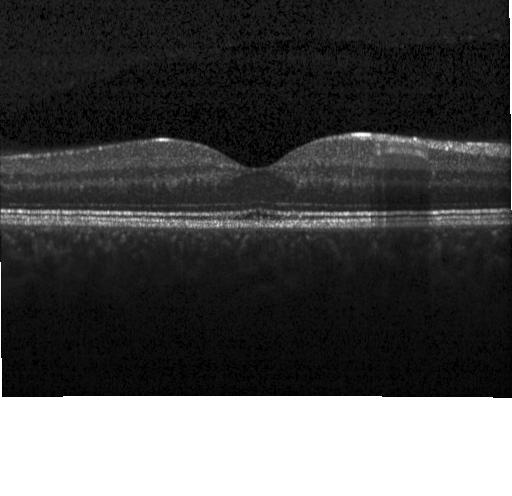
Diagnosis: neither choroidal neovascularization, diabetic macular edema, nor drusen.